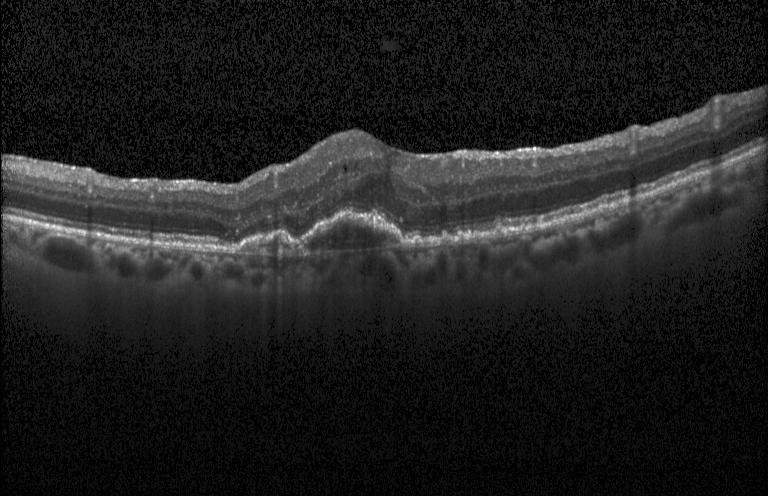
Optical coherence tomography B-scan.
Diagnosis: CNV.